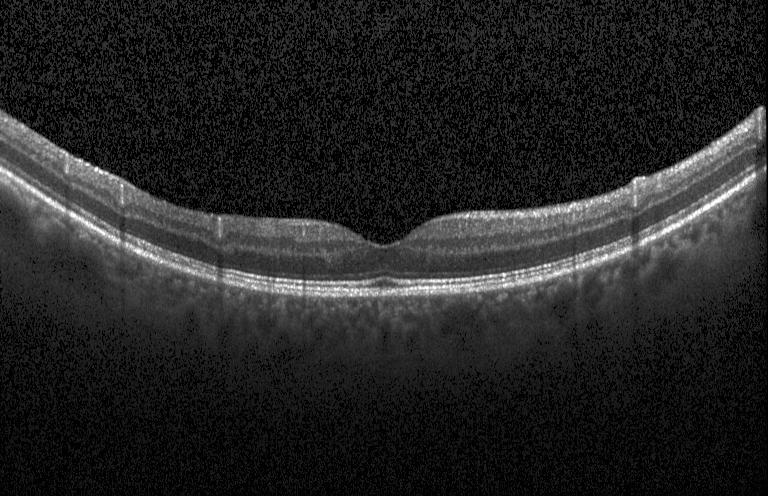

Retinal OCT cross-section; spectral-domain optical coherence tomography; Heidelberg Spectralis
Finding: no choroidal neovascularization, diabetic macular edema, or drusen.